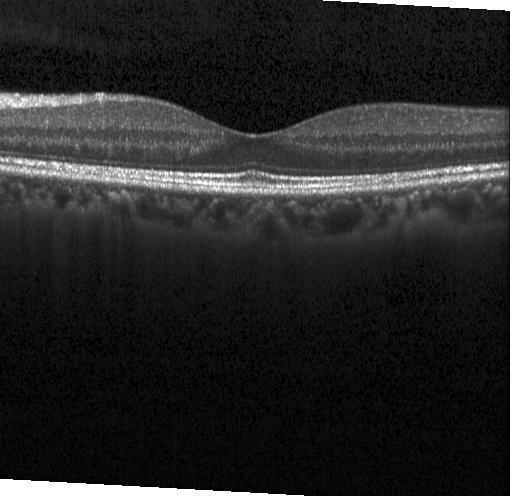

Diagnosis: no CNV, DME, or drusen.